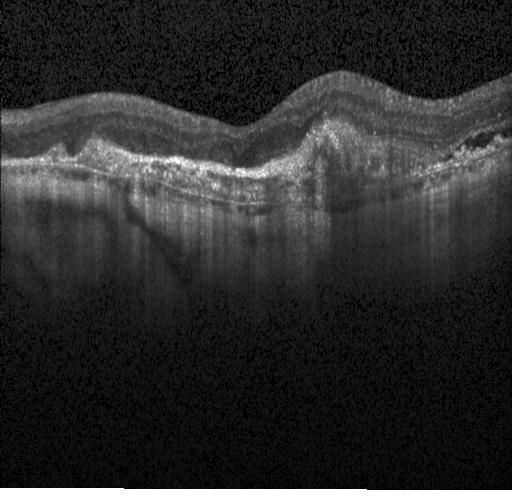
Optical coherence tomography B-scan.
The scan shows a choroidal neovascular membrane.